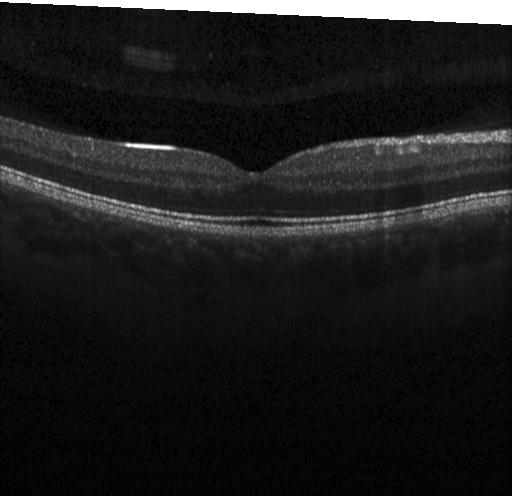

Acquired on a Heidelberg Spectralis. Spectral-domain OCT. Retinal OCT B-scan
The scan shows no choroidal neovascularization, no diabetic macular edema, and no drusen.